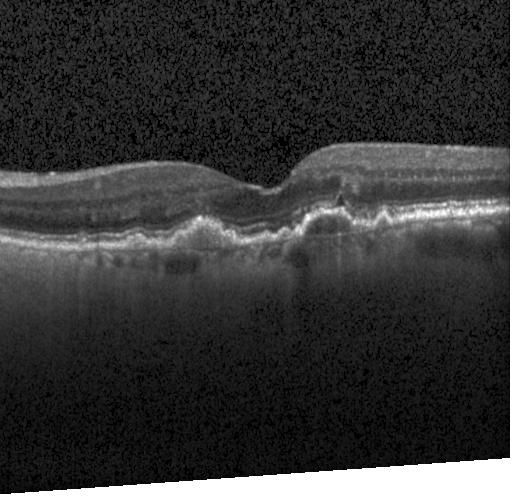
Optical coherence tomography B-scan.
CNV.